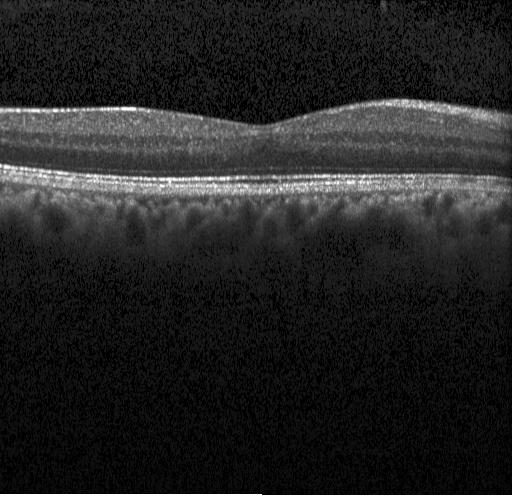
Optical coherence tomography B-scan; SD-OCT; macular scan.
Finding: no evidence of choroidal neovascularization, diabetic macular edema, or drusen.